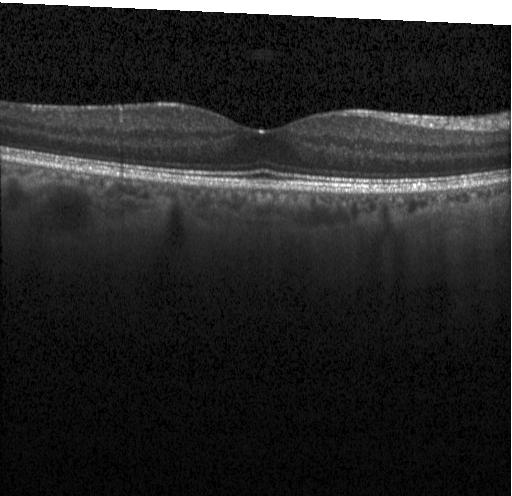

Retinal OCT B-scan. Finding: no evidence of CNV, DME, or drusen.